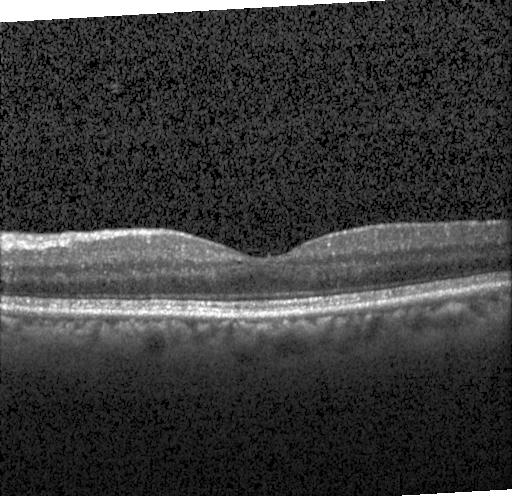 Neither choroidal neovascularization, diabetic macular edema, nor drusen.